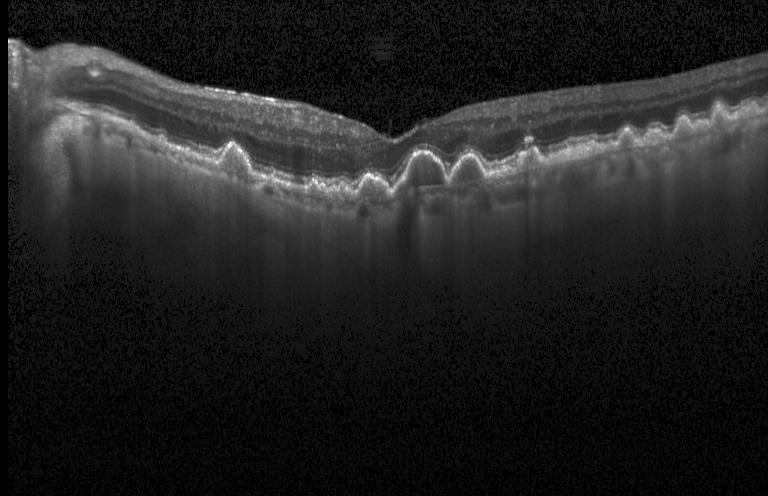

Acquired on a Heidelberg Spectralis · spectral-domain optical coherence tomography · through the macula · optical coherence tomography scan.
Impression: multiple drusen.